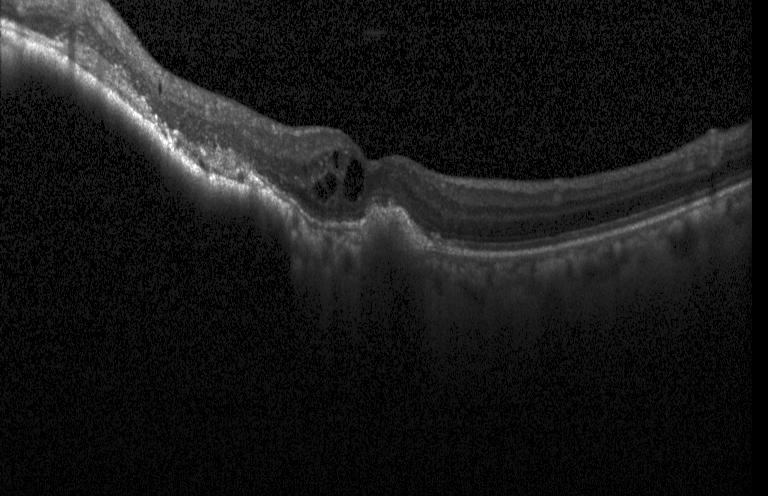
Centered on the fovea. Spectral-domain optical coherence tomography. Optical coherence tomography B-scan
Finding: choroidal neovascularization (CNV).